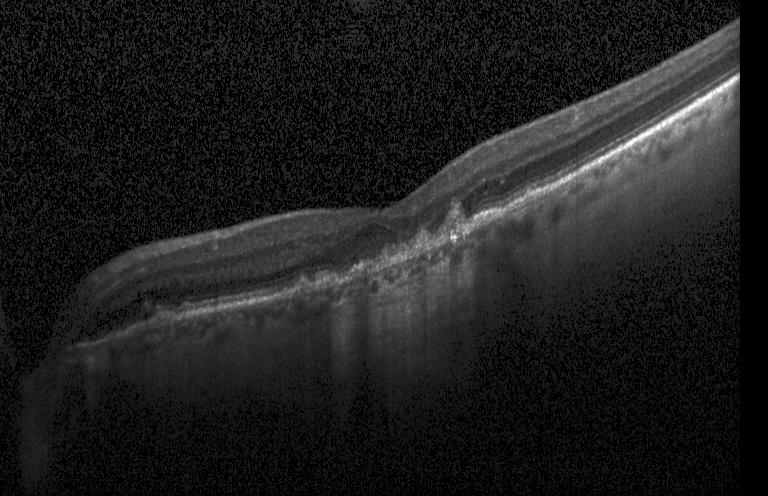
OCT line scan · horizontal scan through the fovea · spectral-domain optical coherence tomography.
Impression: CNV.